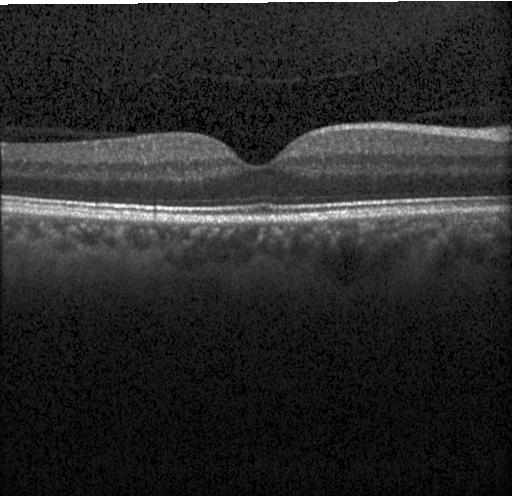
OCT line scan.
Impression: no choroidal neovascularization, no diabetic macular edema, and no drusen.